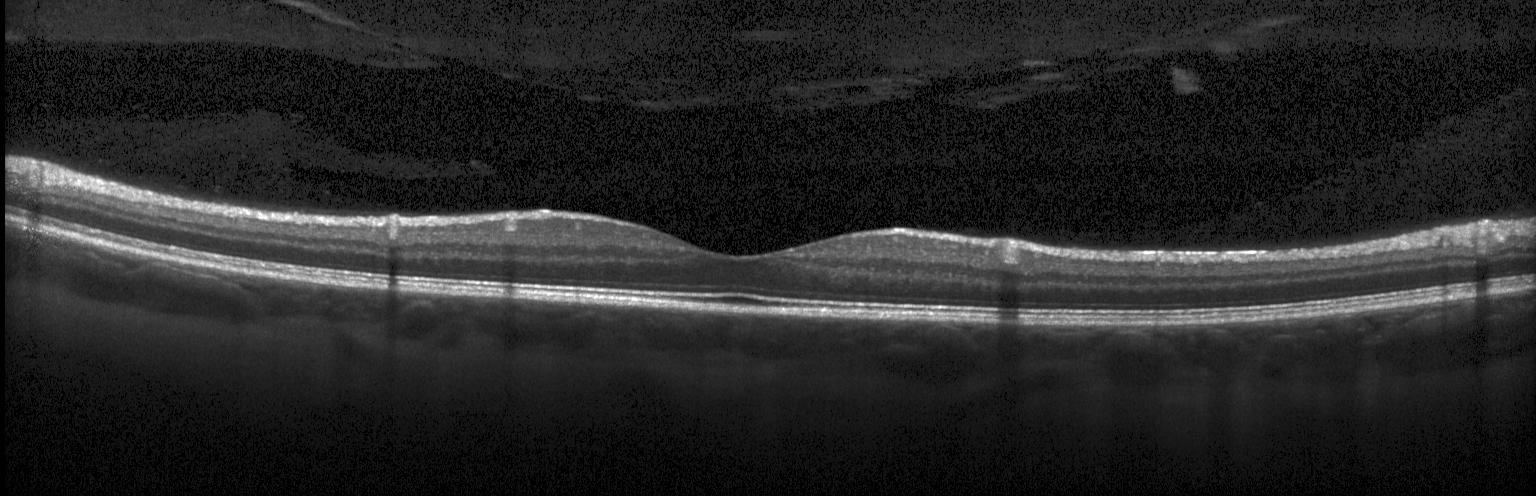

Heidelberg Spectralis · optical coherence tomography B-scan. Finding: no evidence of CNV, DME, or drusen.